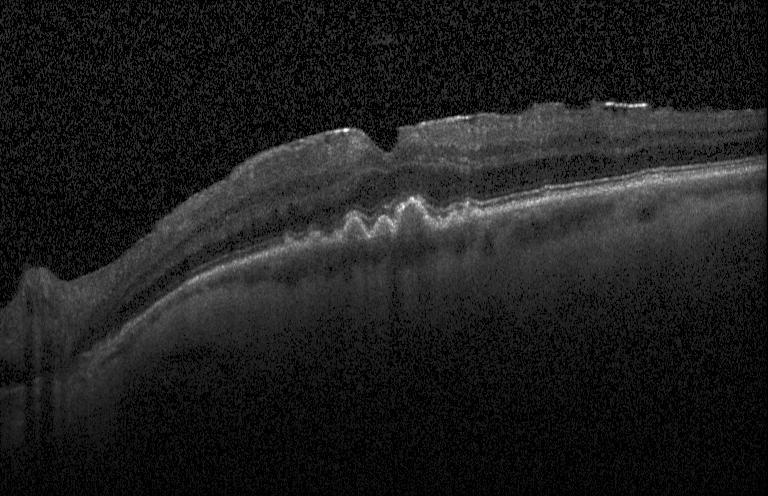
Optical coherence tomography B-scan · acquired on a Heidelberg Spectralis · spectral-domain optical coherence tomography · through the macula.
OCT finding: drusen.